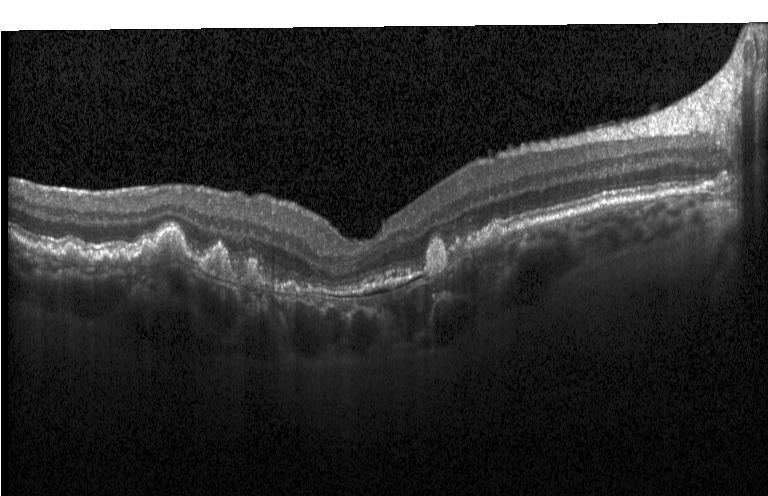 Assessment: CNV.